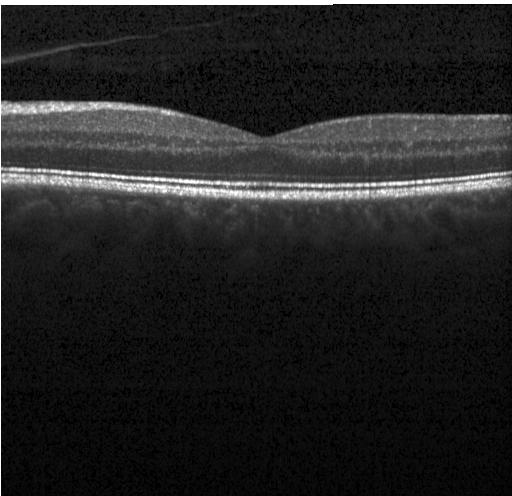

This B-scan demonstrates no evidence of choroidal neovascularization, diabetic macular edema, or drusen.